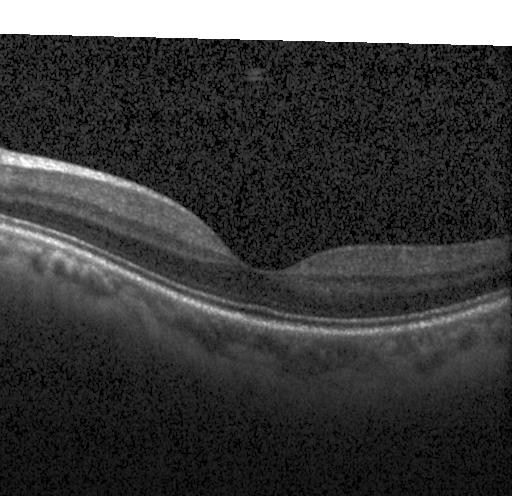

Macular OCT demonstrating no choroidal neovascularization, no diabetic macular edema, and no drusen.